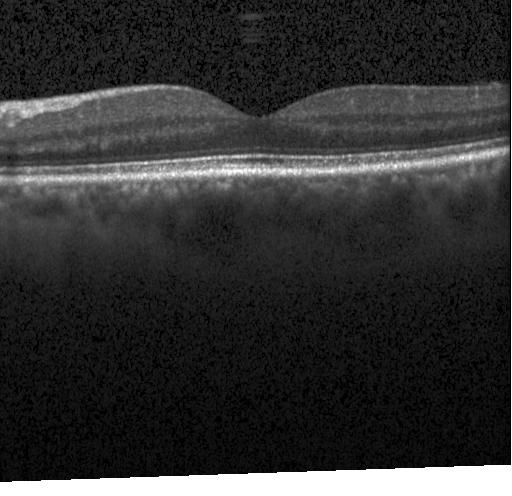 Impression: no choroidal neovascularization, diabetic macular edema, or drusen.